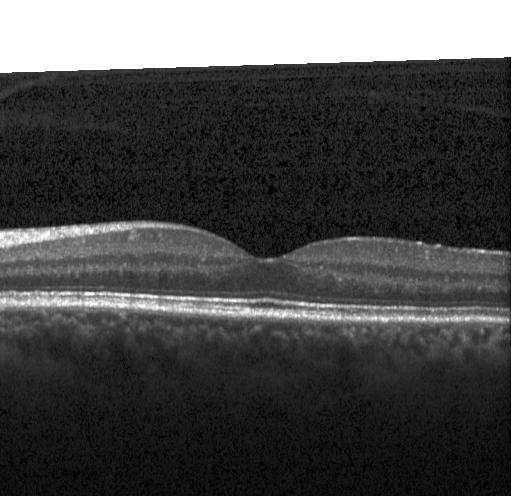

Optical coherence tomography scan. Macular scan. Acquired on a Heidelberg Spectralis — Macular OCT: no CNV, DME, or drusen.